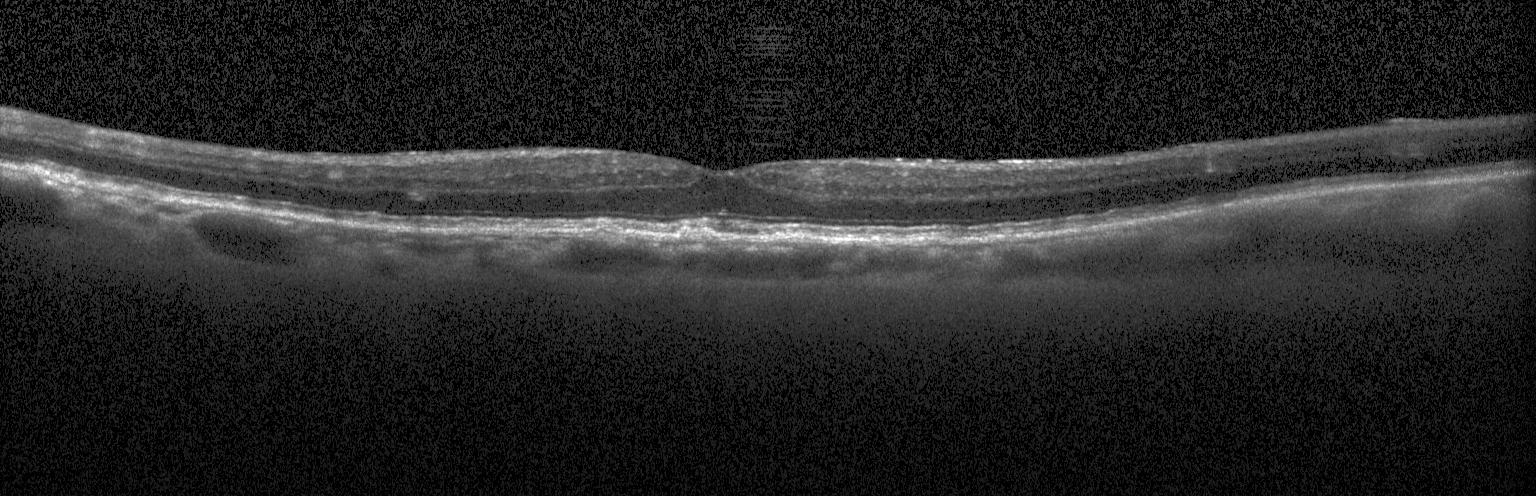
This B-scan demonstrates sub-RPE drusenoid deposits.